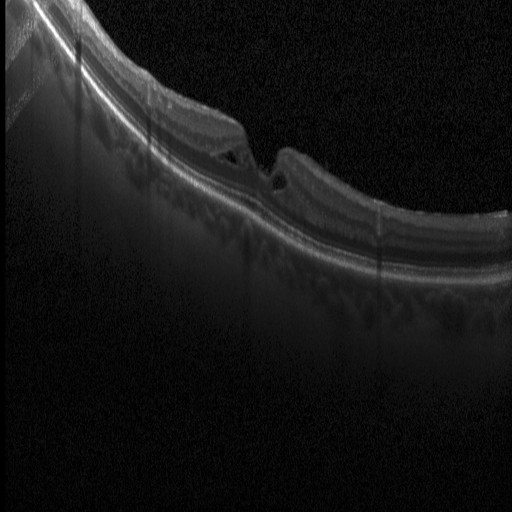

Dx: diabetic macular edema (DME).